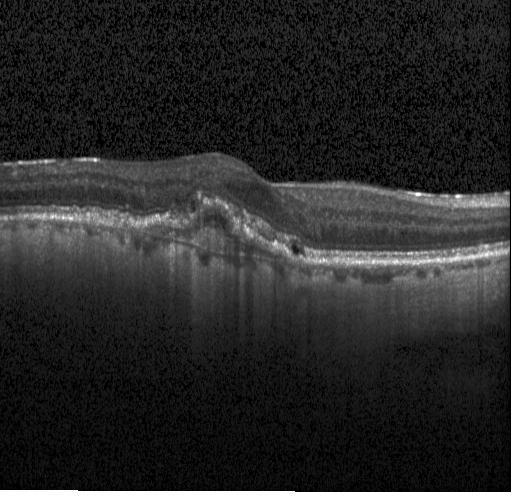

Optical coherence tomography scan; SD-OCT; macular scan — Finding: CNV.